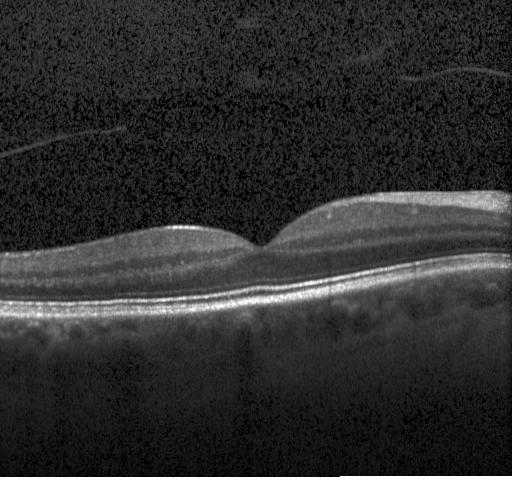
Assessment: neither choroidal neovascularization, diabetic macular edema, nor drusen.